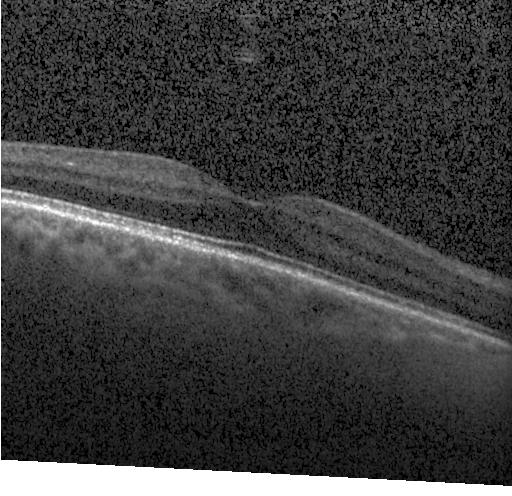

Instrument: Heidelberg Spectralis, through the macula, spectral-domain optical coherence tomography, retinal OCT cross-section. Finding: neither choroidal neovascularization, diabetic macular edema, nor drusen.